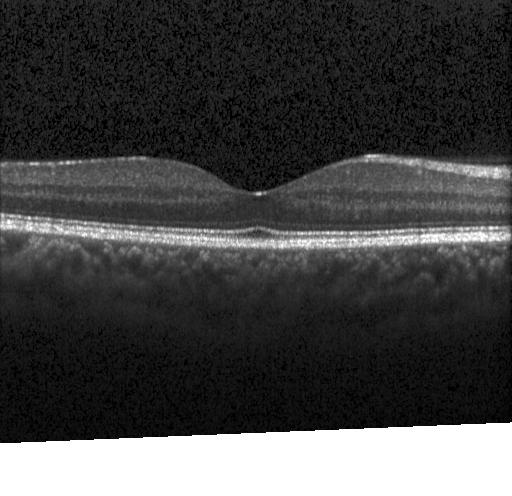 OCT B-scan — Diagnosis: no CNV, no DME, and no drusen.